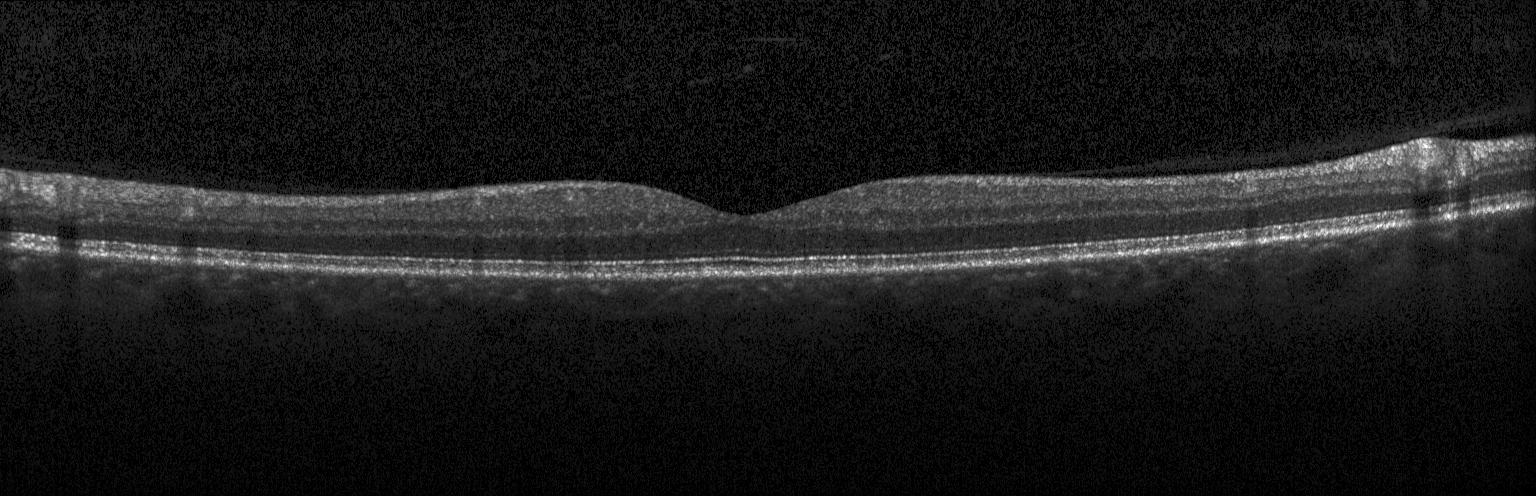
Assessment: no choroidal neovascularization, diabetic macular edema, or drusen.